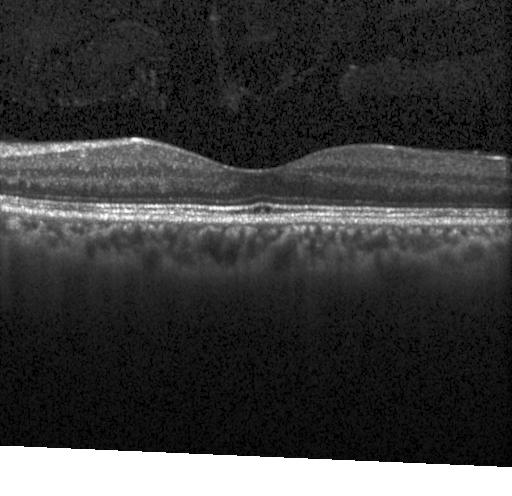
OCT line scan. Through the macula. Spectral-domain optical coherence tomography.
Macular OCT: no evidence of CNV, DME, or drusen.